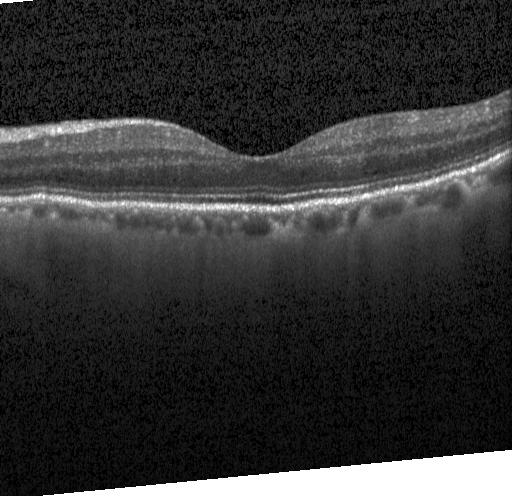 Optical coherence tomography B-scan.
Diagnosis: no choroidal neovascularization, no diabetic macular edema, and no drusen.